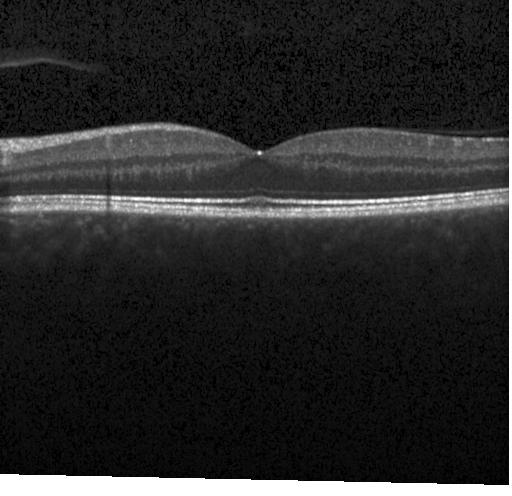
Retinal OCT cross-section showing no CNV, no DME, and no drusen.